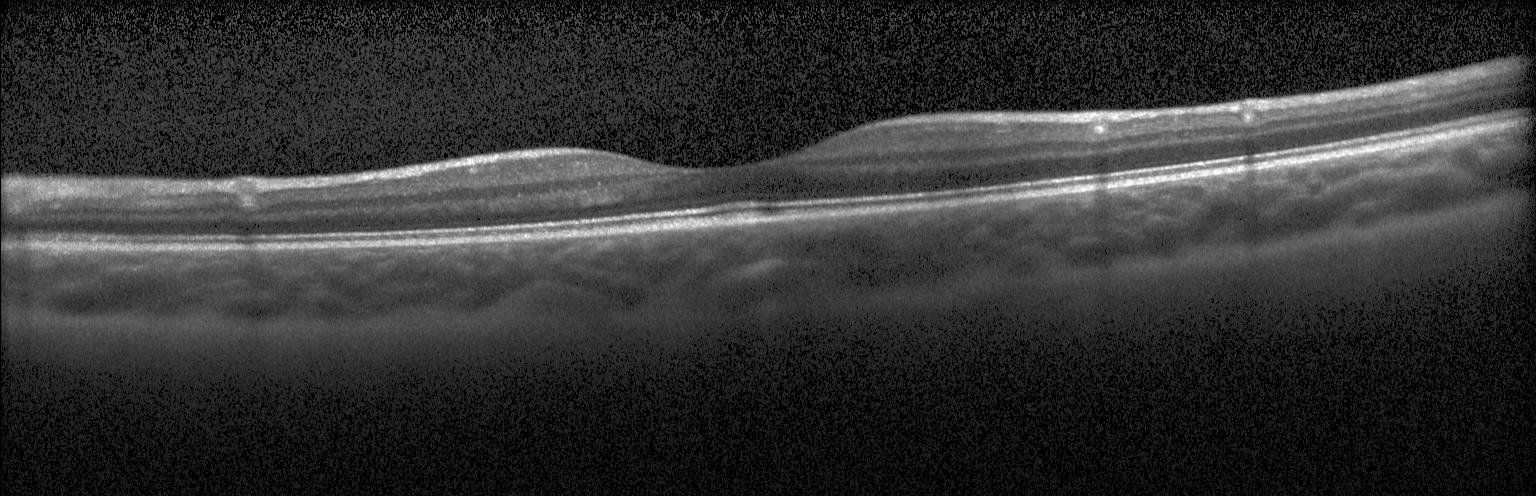 Diagnosis: no choroidal neovascularization, no diabetic macular edema, and no drusen.